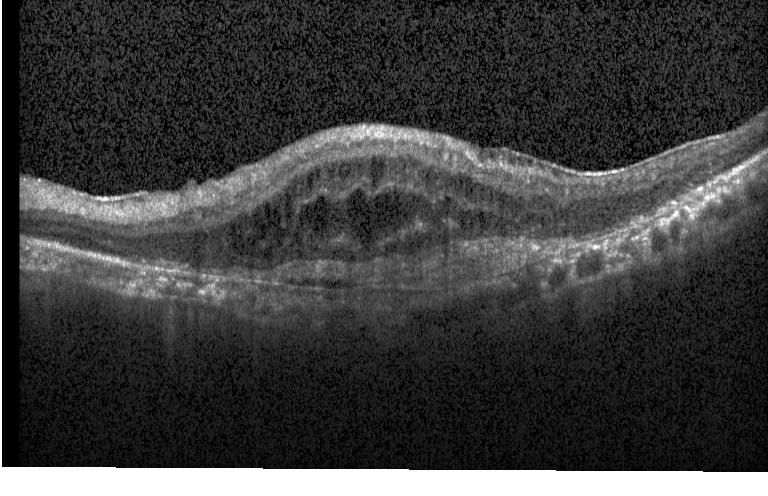 Retinal OCT B-scan · SD-OCT.
OCT finding: a choroidal neovascular membrane.